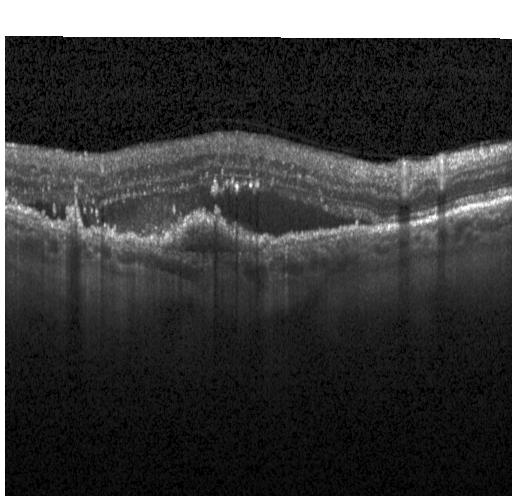
This B-scan demonstrates CNV.